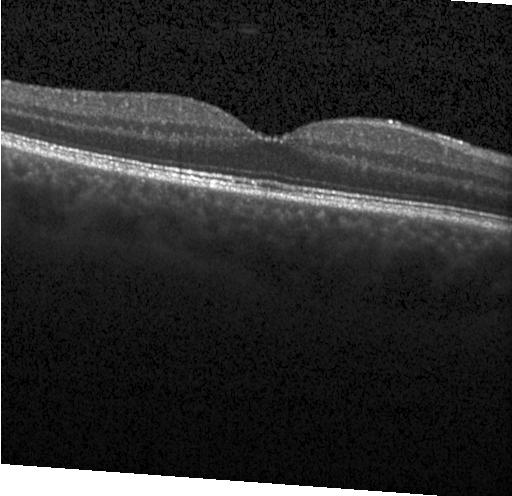 OCT finding: no evidence of choroidal neovascularization, diabetic macular edema, or drusen.